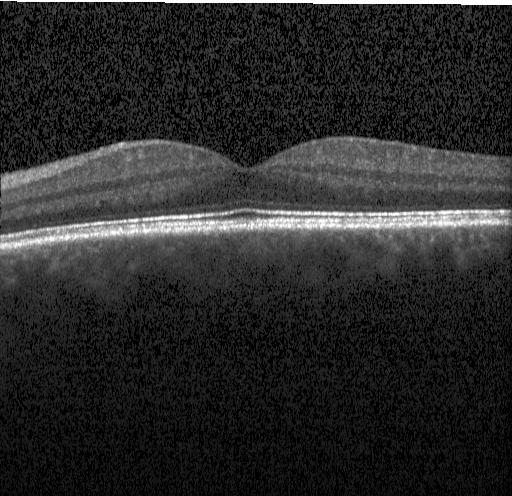 Heidelberg Spectralis OCT system, spectral-domain OCT, fovea-centered, optical coherence tomography scan. Dx: no choroidal neovascularization, no diabetic macular edema, and no drusen.